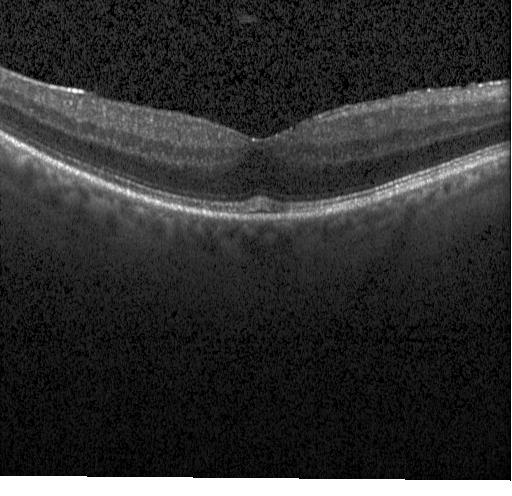

Optical coherence tomography B-scan. SD-OCT — No choroidal neovascularization, no diabetic macular edema, and no drusen.